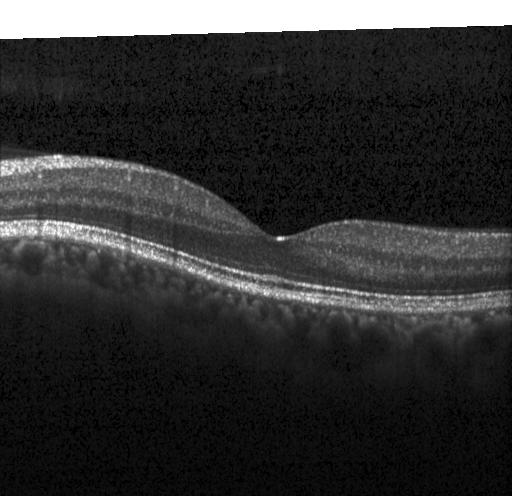 Macular OCT: no choroidal neovascularization, diabetic macular edema, or drusen.